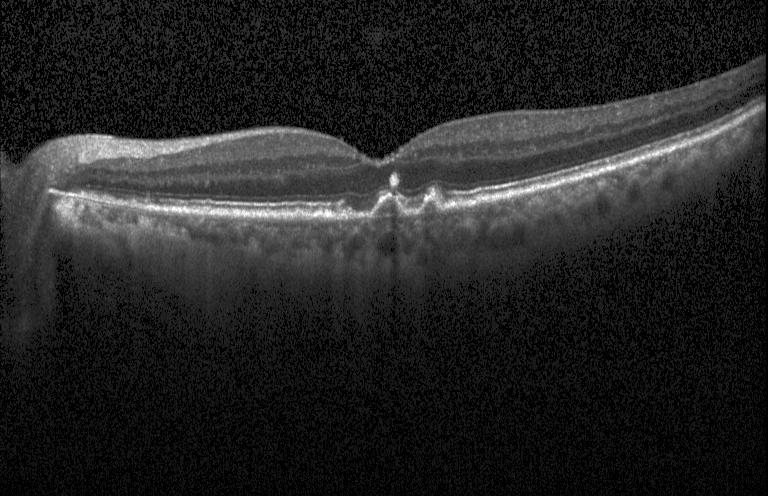 Macular OCT demonstrating sub-RPE drusenoid deposits.